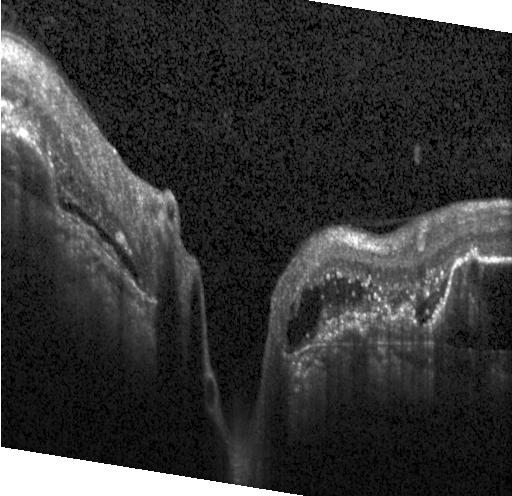

OCT line scan, centered on the fovea
Impression: CNV.